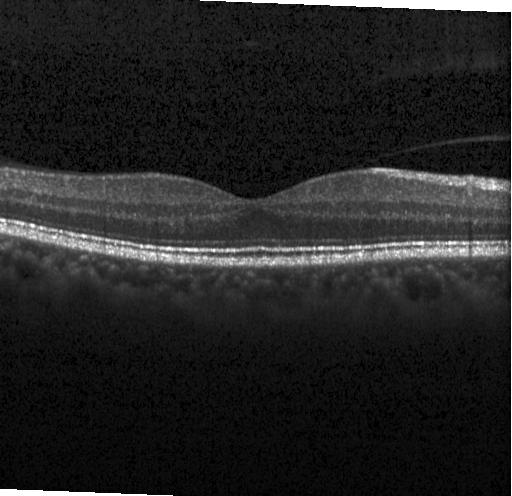 Spectral-domain optical coherence tomography · acquired on a Heidelberg Spectralis · OCT B-scan · horizontal scan through the fovea
Diagnosis: no choroidal neovascularization, diabetic macular edema, or drusen.